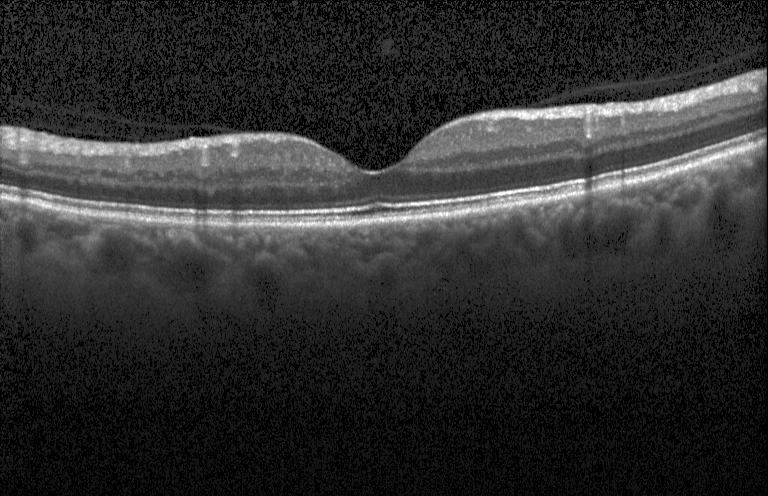
Neither CNV, DME, nor drusen.